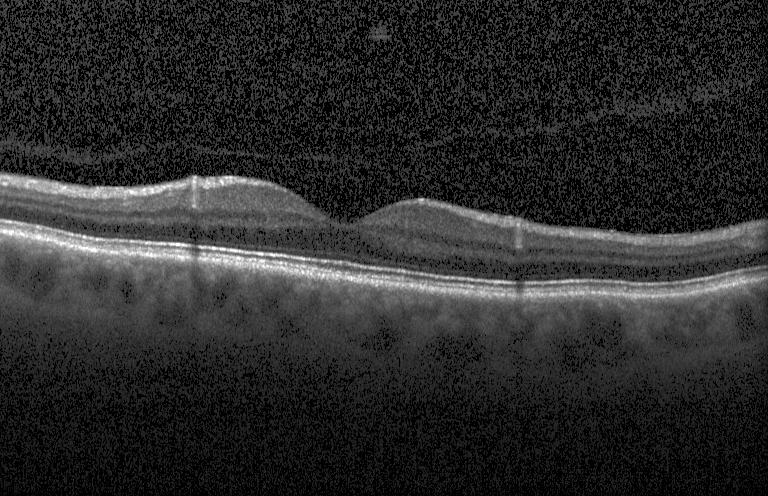 Fovea-centered. Retinal OCT cross-section
Assessment: no CNV, DME, or drusen.